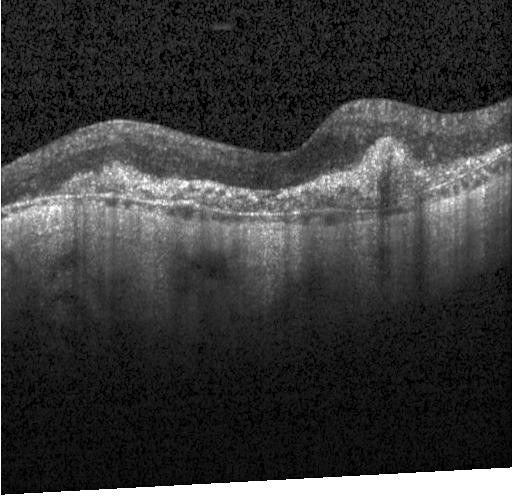 Fovea-centered, optical coherence tomography scan, spectral-domain OCT
The scan shows a choroidal neovascular membrane.